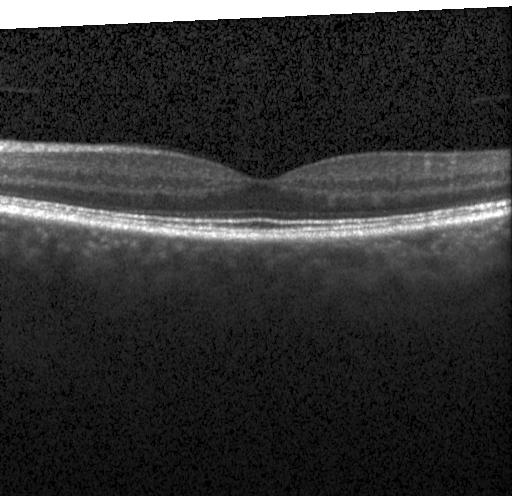 Impression: neither CNV, DME, nor drusen.